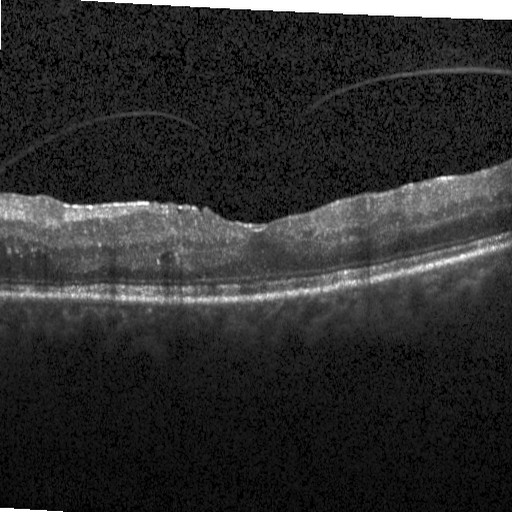
Spectral-domain optical coherence tomography; retinal OCT cross-section; Heidelberg Spectralis; macular scan
This B-scan demonstrates diabetic macular edema (DME).